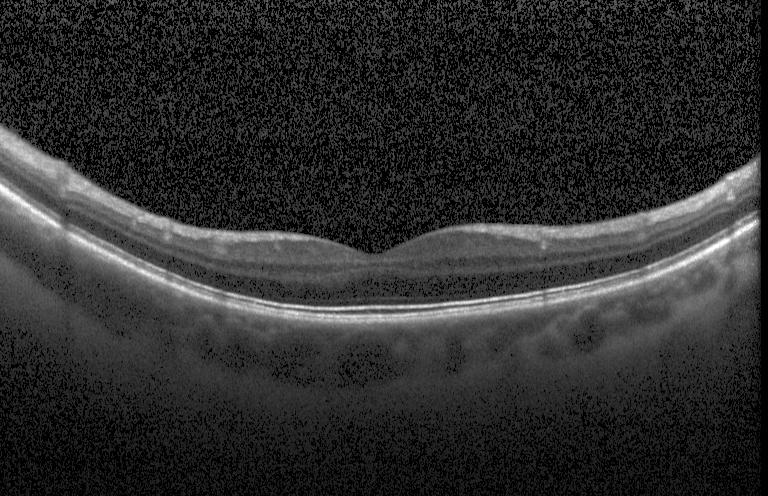

SD-OCT, OCT B-scan — Impression: no choroidal neovascularization, no diabetic macular edema, and no drusen.